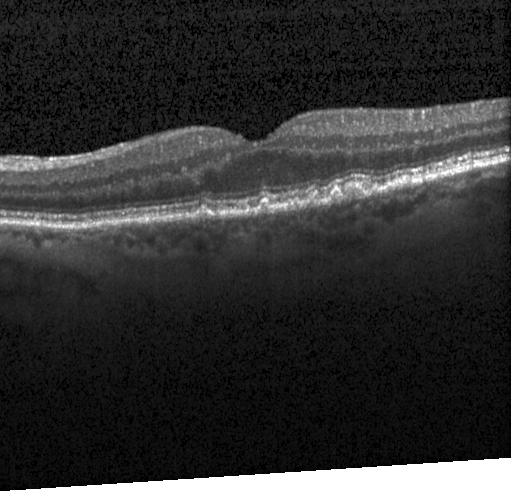

Macular OCT: sub-RPE drusenoid deposits.